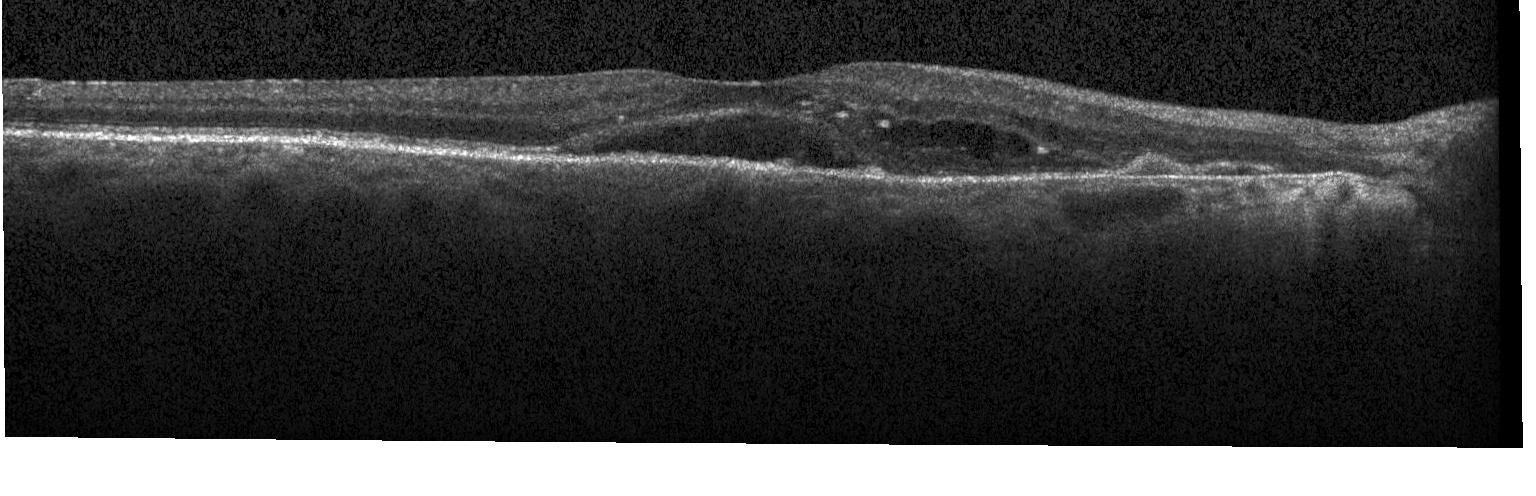 Macular OCT demonstrating a choroidal neovascular membrane.